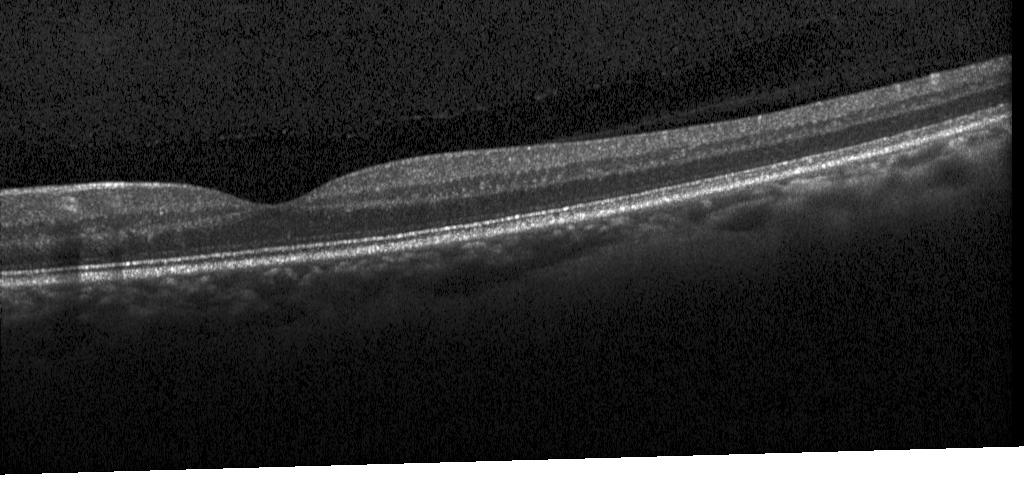

OCT line scan · Heidelberg Spectralis OCT system · spectral-domain OCT.
Diagnosis: no choroidal neovascularization, diabetic macular edema, or drusen.